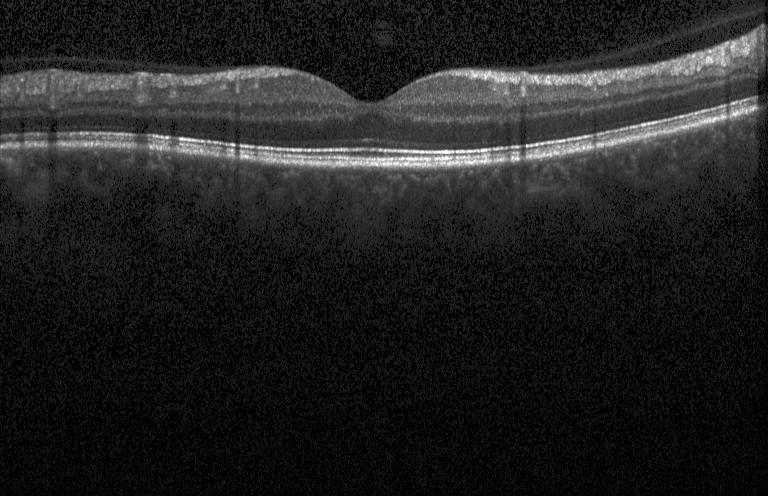 SD-OCT; optical coherence tomography B-scan; Heidelberg Spectralis. OCT finding: no choroidal neovascularization, diabetic macular edema, or drusen.